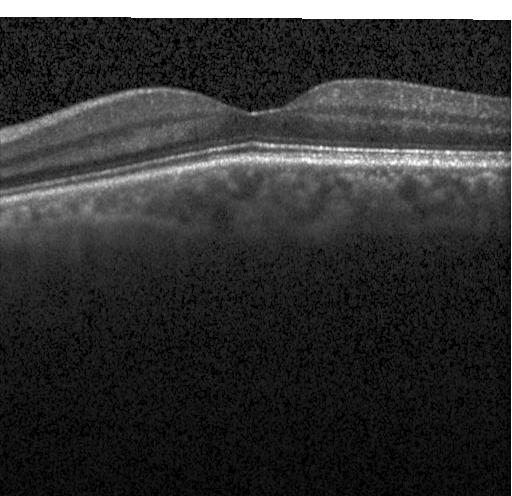

OCT B-scan
This B-scan demonstrates no CNV, no DME, and no drusen.